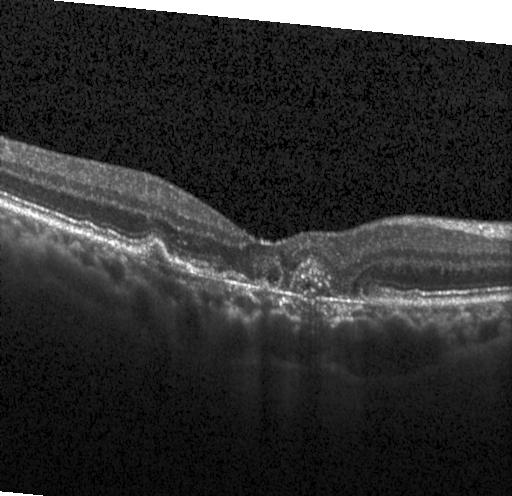

CNV.